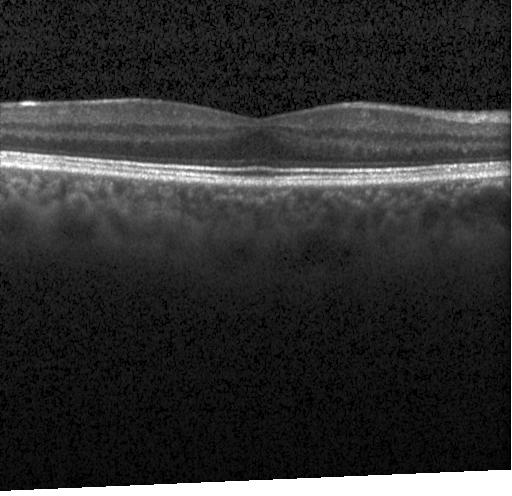 Heidelberg Spectralis · centered on the fovea · spectral-domain optical coherence tomography · optical coherence tomography scan
Finding: no evidence of choroidal neovascularization, diabetic macular edema, or drusen.